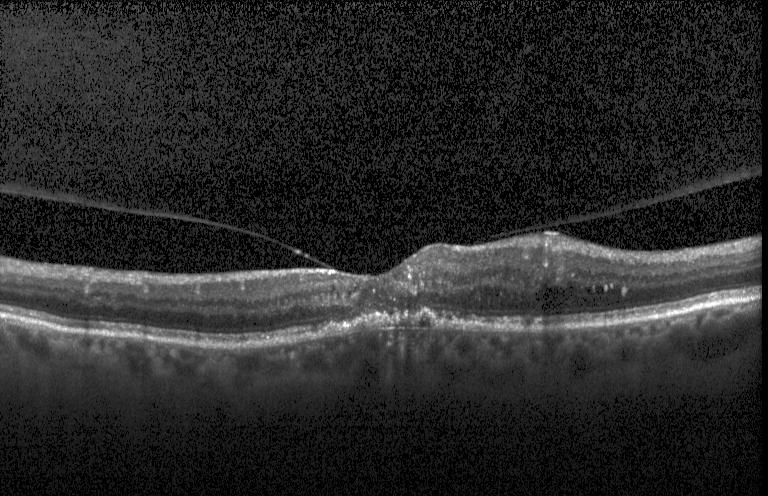 Horizontal scan through the fovea; retinal OCT cross-section; spectral-domain OCT. OCT finding: a choroidal neovascular membrane.